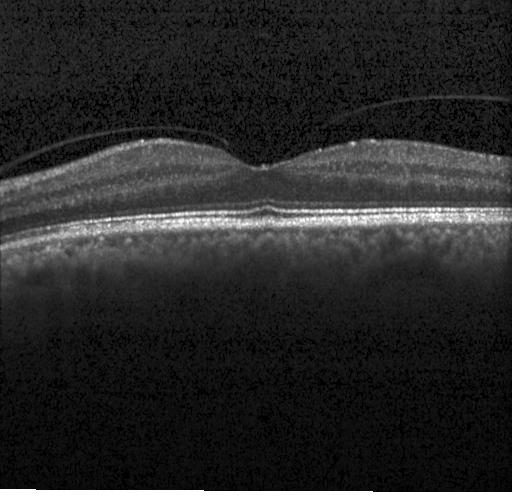 Acquired on a Heidelberg Spectralis. Retinal OCT cross-section
Diagnosis: no choroidal neovascularization, diabetic macular edema, or drusen.